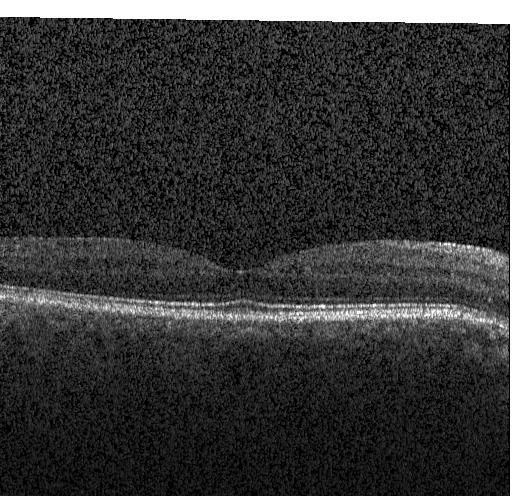
Optical coherence tomography scan — Finding: no CNV, no DME, and no drusen.